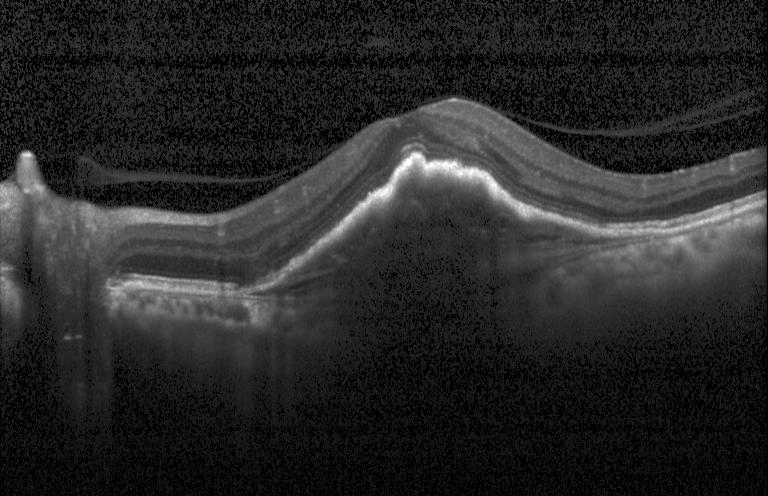

Heidelberg Spectralis; fovea-centered; OCT B-scan
Finding: a choroidal neovascular membrane.